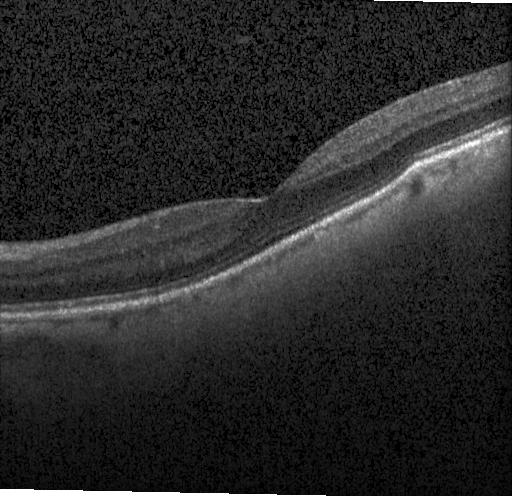
Spectral-domain optical coherence tomography, centered on the fovea, optical coherence tomography B-scan, acquired on a Heidelberg Spectralis
OCT finding: no choroidal neovascularization, no diabetic macular edema, and no drusen.